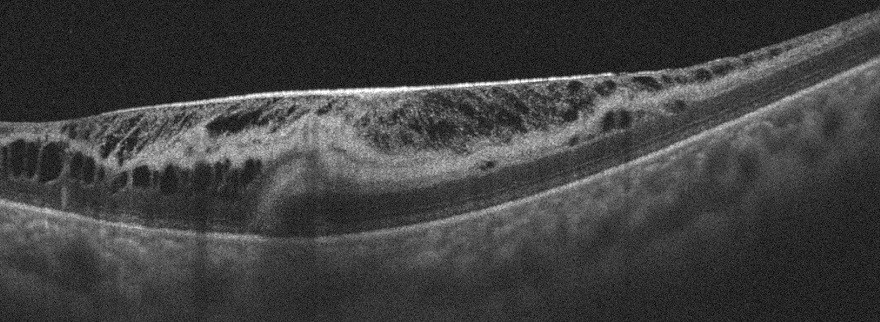
Retinal OCT cross-section. Impression: ERM.